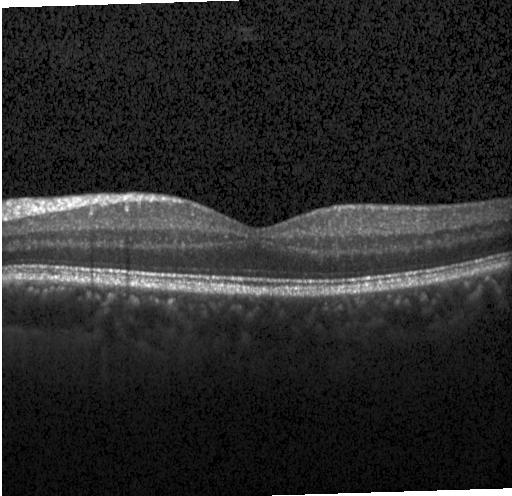
Macular OCT: no choroidal neovascularization, no diabetic macular edema, and no drusen.